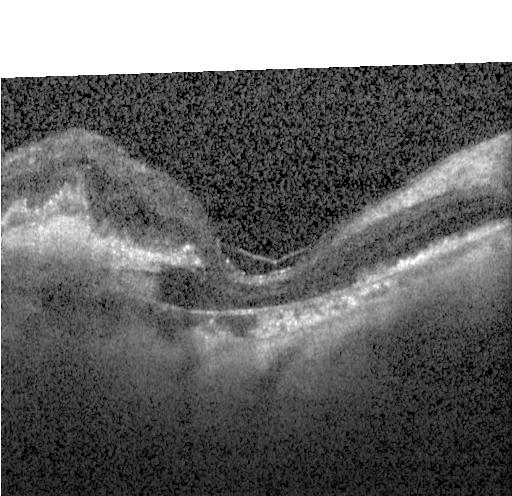
Retinal OCT cross-section. Finding: a choroidal neovascular membrane.